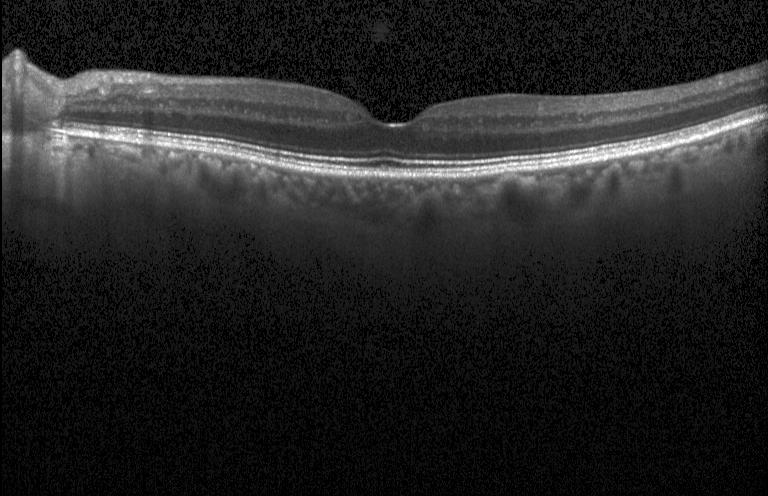 SD-OCT, horizontal scan through the fovea, acquired on a Heidelberg Spectralis, optical coherence tomography scan. Diagnosis: no evidence of CNV, DME, or drusen.